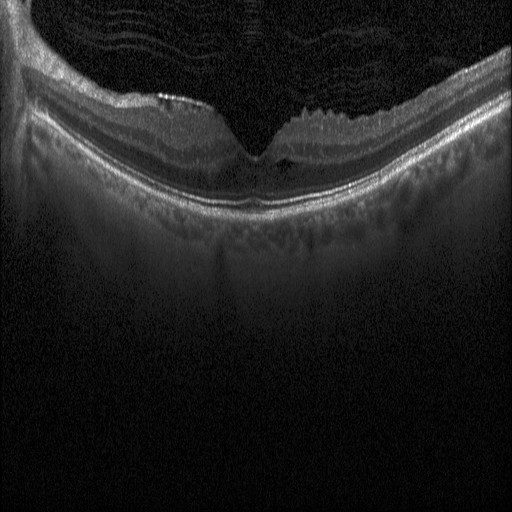 Optical coherence tomography scan
Finding: diabetic macular edema.